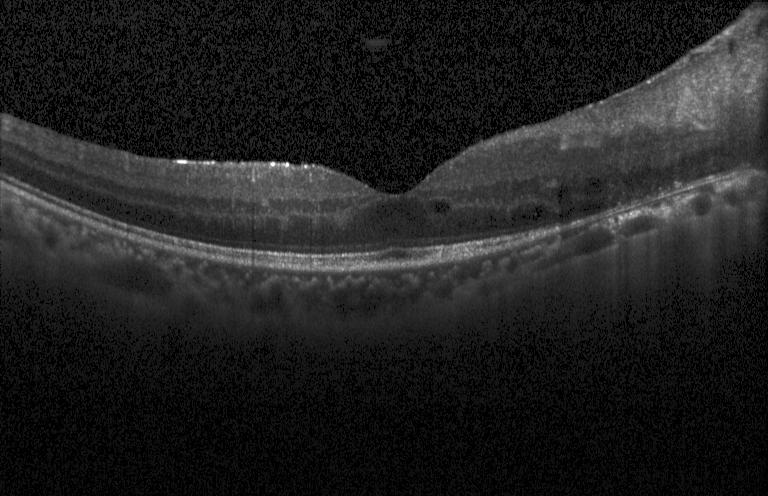

Spectral-domain OCT, optical coherence tomography scan
Diabetic macular edema.